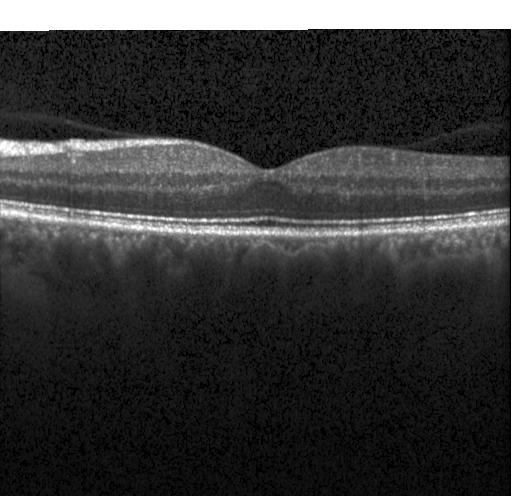 OCT line scan. Macular scan. Assessment: no evidence of choroidal neovascularization, diabetic macular edema, or drusen.